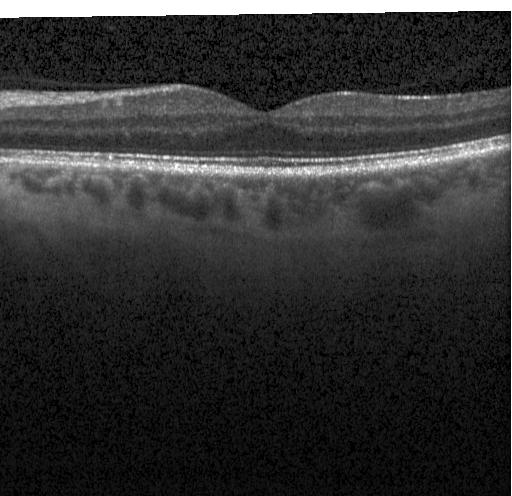
Optical coherence tomography scan. The scan shows no CNV, no DME, and no drusen.